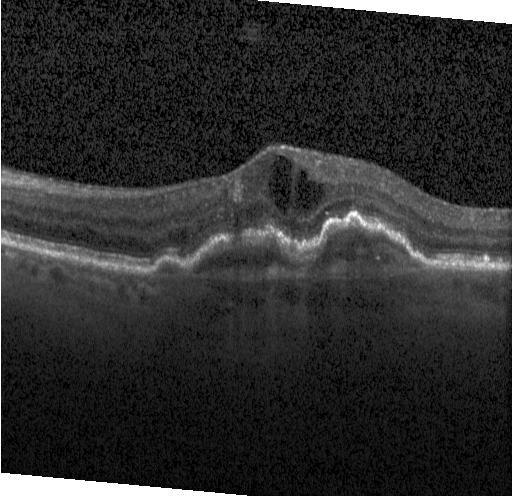
OCT finding: choroidal neovascularization.